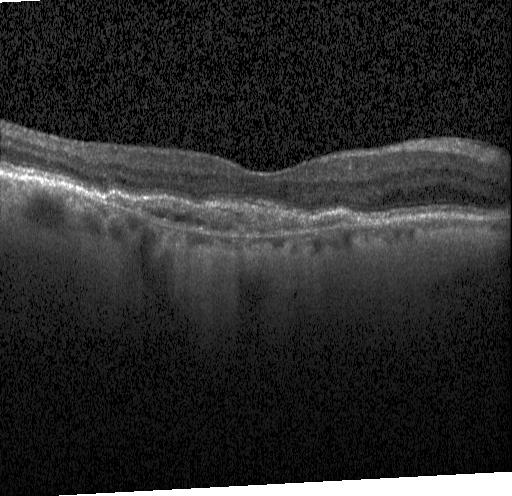 Retinal OCT cross-section showing choroidal neovascularization.